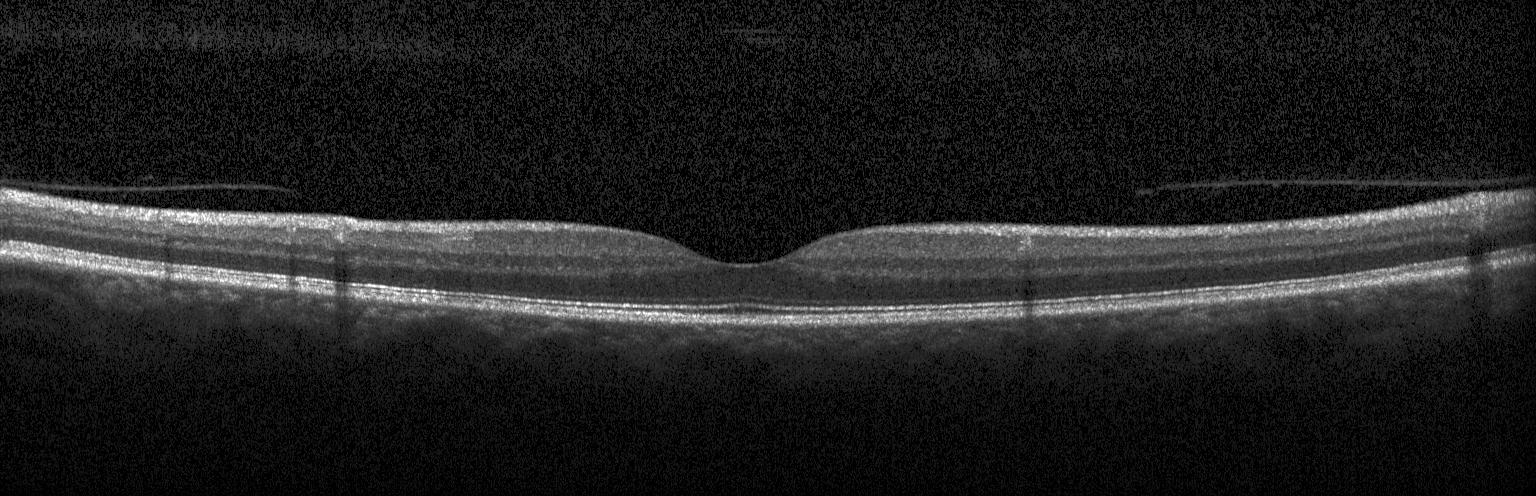 Spectral-domain optical coherence tomography · OCT line scan · macular scan · instrument: Heidelberg Spectralis.
Impression: no CNV, DME, or drusen.